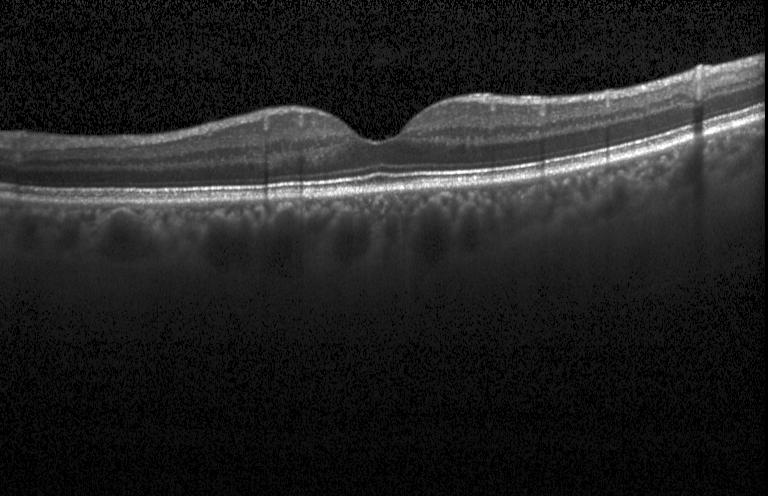 Horizontal scan through the fovea; retinal OCT B-scan; Heidelberg Spectralis OCT system — Impression: neither choroidal neovascularization, diabetic macular edema, nor drusen.